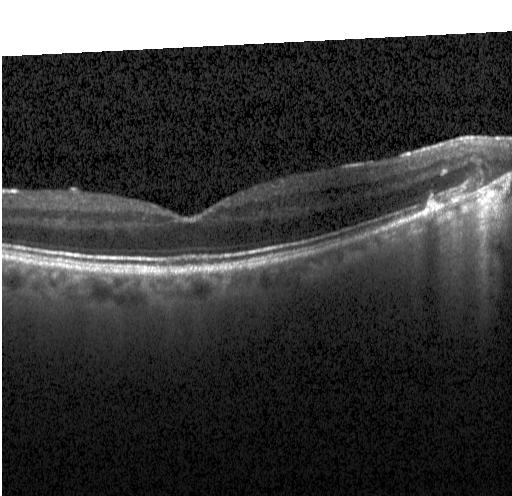 Impression: neither choroidal neovascularization, diabetic macular edema, nor drusen.